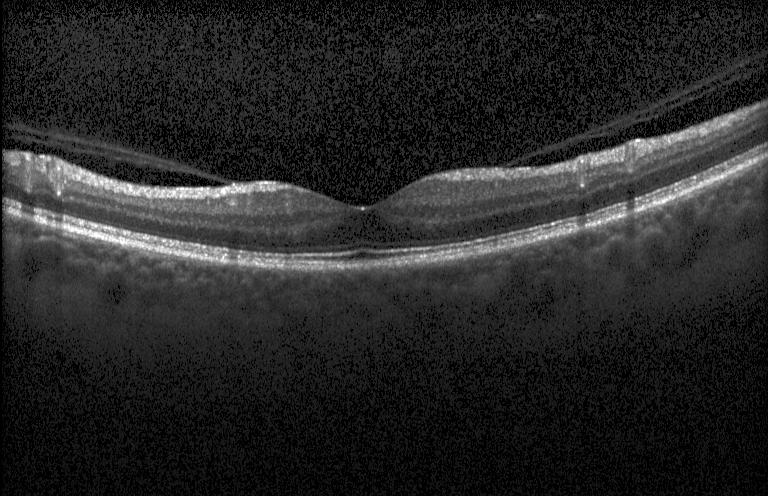

Spectral-domain optical coherence tomography, macular scan, optical coherence tomography scan, acquired on a Heidelberg Spectralis. The scan shows no CNV, no DME, and no drusen.